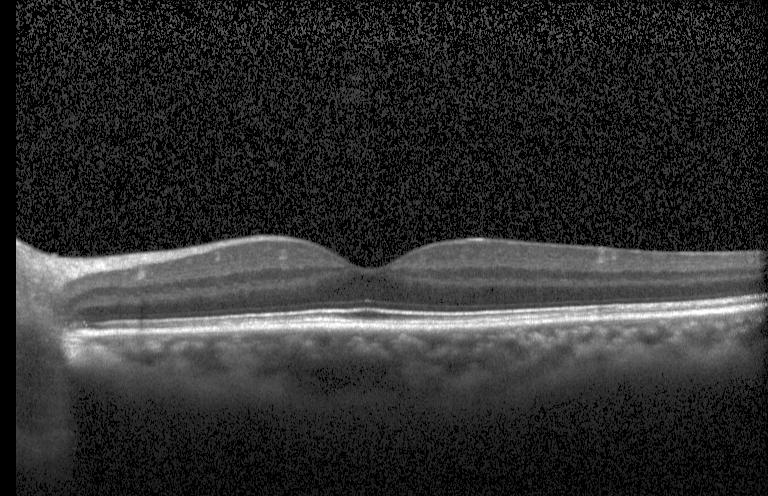

Heidelberg Spectralis OCT system. SD-OCT. Centered on the fovea. OCT line scan — Impression: no evidence of choroidal neovascularization, diabetic macular edema, or drusen.